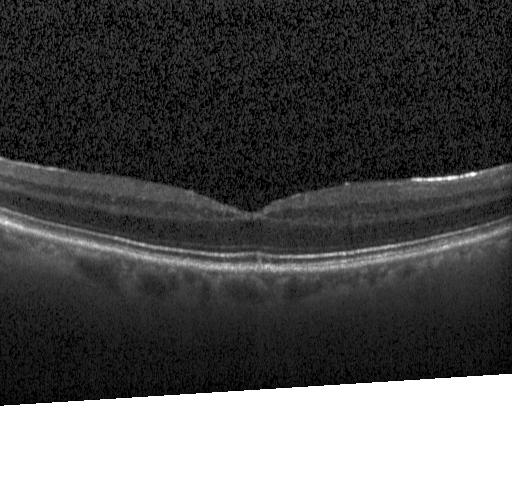

Retinal OCT cross-section.
Impression: no CNV, no DME, and no drusen.